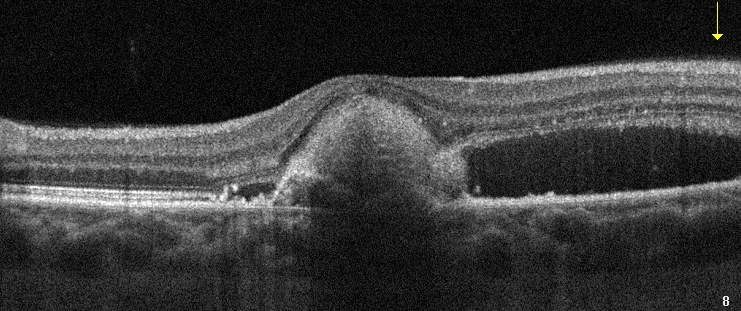
Retinal OCT B-scan. Impression: age-related macular degeneration (AMD).